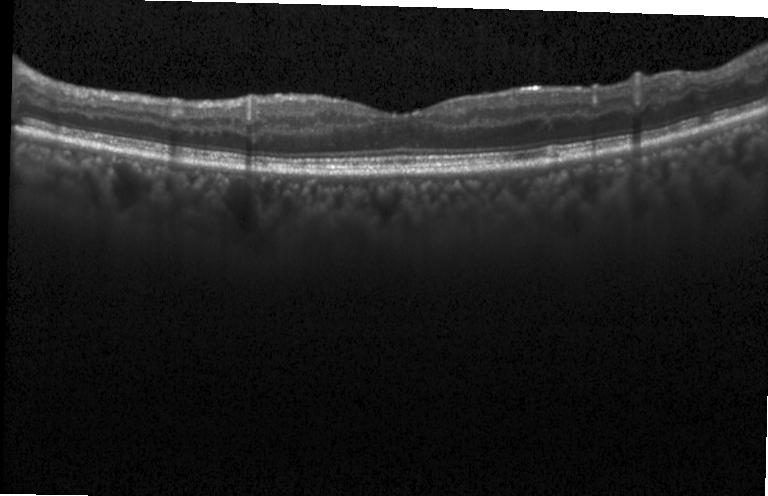

Diagnosis: no CNV, DME, or drusen.